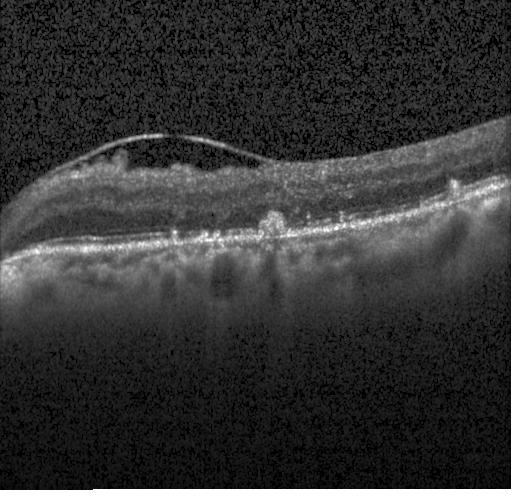 Impression: choroidal neovascularization (CNV).